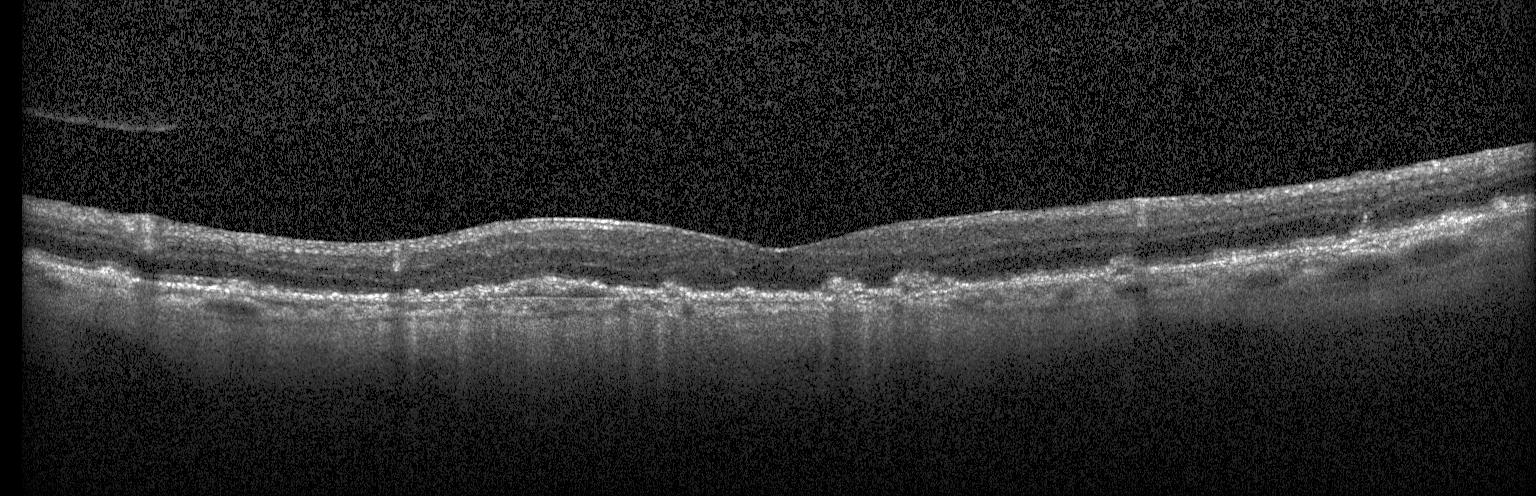
Diagnosis: choroidal neovascularization.